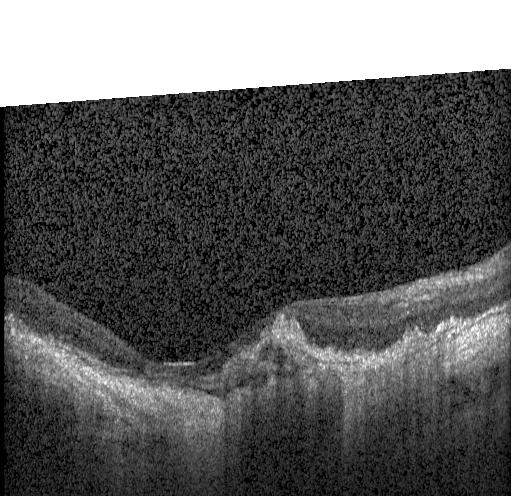

OCT finding: choroidal neovascularization (CNV).